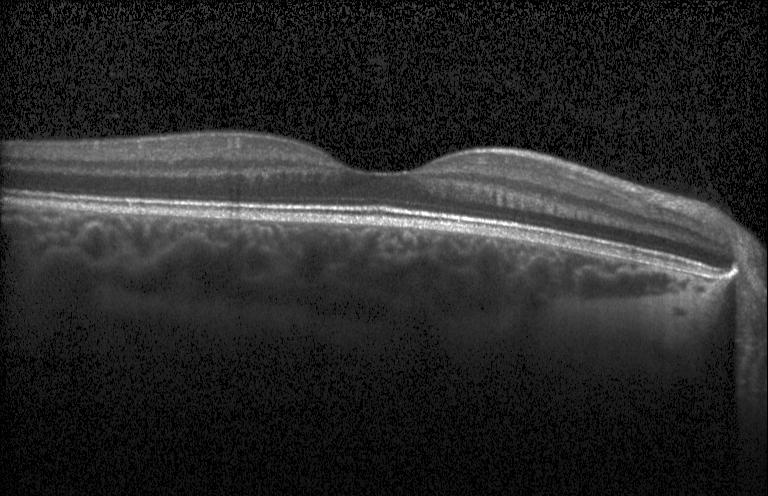 Optical coherence tomography B-scan. Impression: neither choroidal neovascularization, diabetic macular edema, nor drusen.